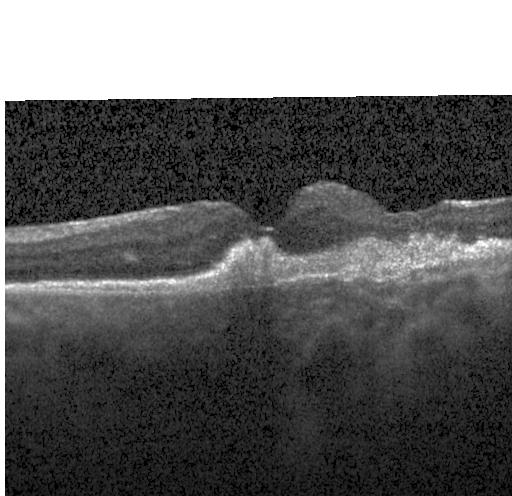

Spectral-domain optical coherence tomography. Optical coherence tomography B-scan.
Impression: choroidal neovascularization.